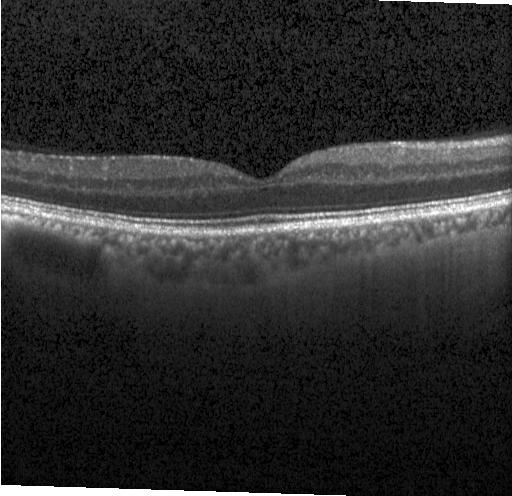 Assessment: no evidence of choroidal neovascularization, diabetic macular edema, or drusen.